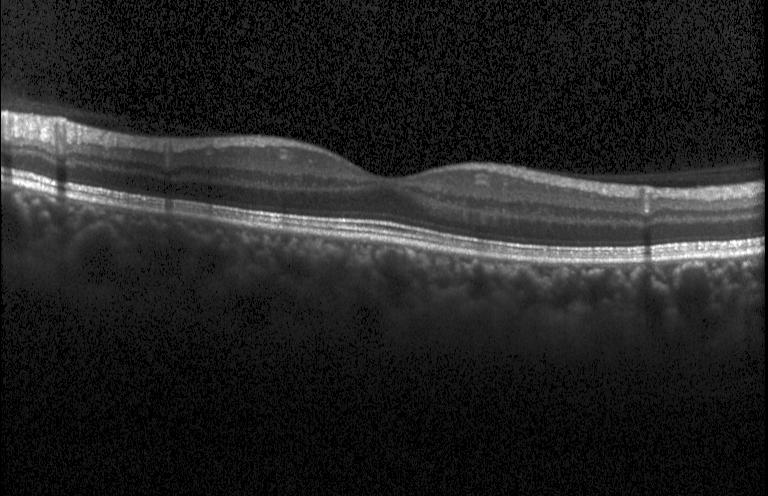

Fovea-centered · spectral-domain optical coherence tomography · OCT B-scan
Finding: neither choroidal neovascularization, diabetic macular edema, nor drusen.